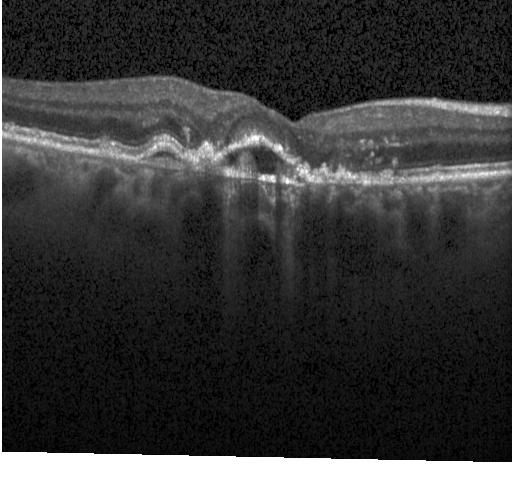 Spectral-domain optical coherence tomography, OCT B-scan, instrument: Heidelberg Spectralis, macular scan.
This B-scan demonstrates choroidal neovascularization.